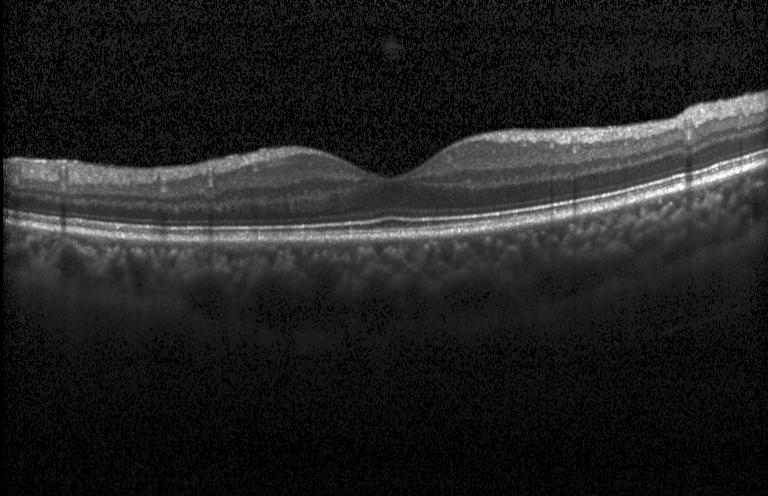 Centered on the fovea · OCT B-scan · SD-OCT — Finding: no choroidal neovascularization, no diabetic macular edema, and no drusen.